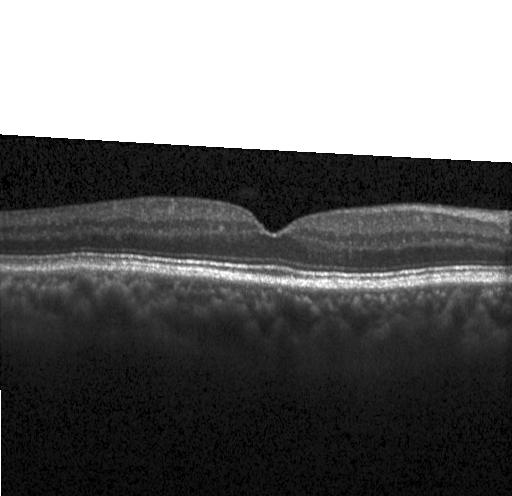 Through the macula · OCT line scan. Diagnosis: no choroidal neovascularization, no diabetic macular edema, and no drusen.